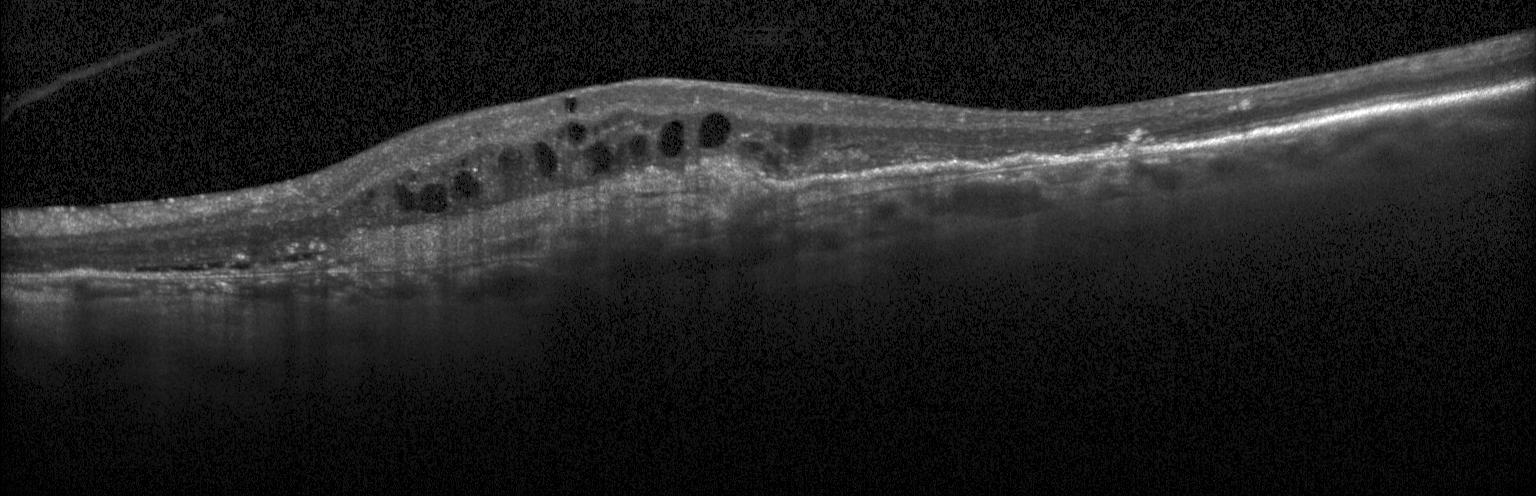

The scan shows a choroidal neovascular membrane.